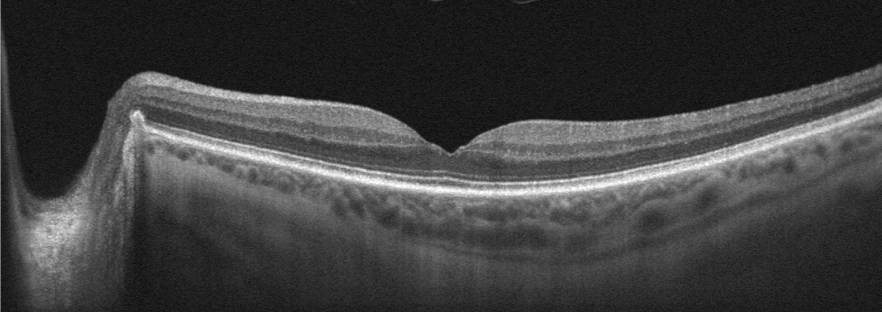
Finding: no AMD, DME, ERM, RAO, RVO, or VID.